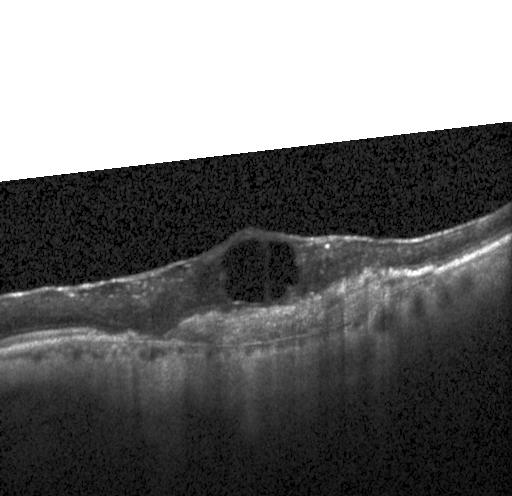

Assessment: a choroidal neovascular membrane.